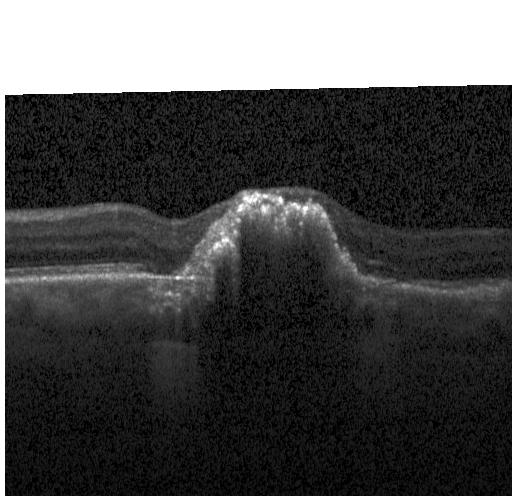
Fovea-centered, Heidelberg Spectralis, optical coherence tomography B-scan — Diagnosis: CNV.